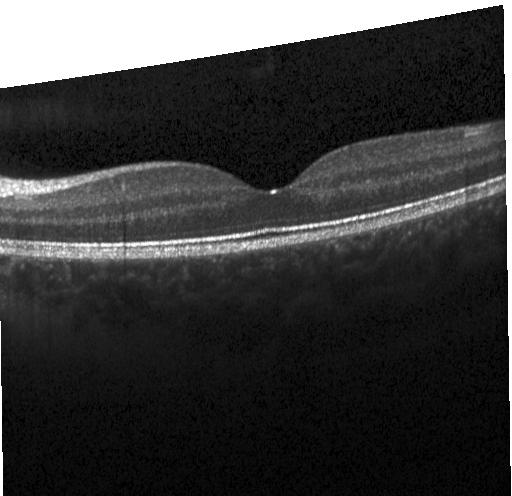

OCT B-scan; Heidelberg Spectralis OCT system; spectral-domain optical coherence tomography; macular scan
This B-scan demonstrates no choroidal neovascularization, no diabetic macular edema, and no drusen.